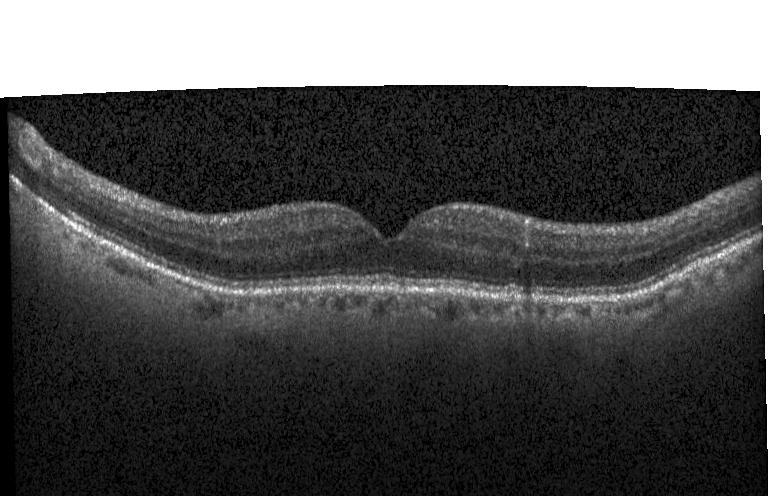
Instrument: Heidelberg Spectralis. Optical coherence tomography B-scan.
Impression: no evidence of choroidal neovascularization, diabetic macular edema, or drusen.